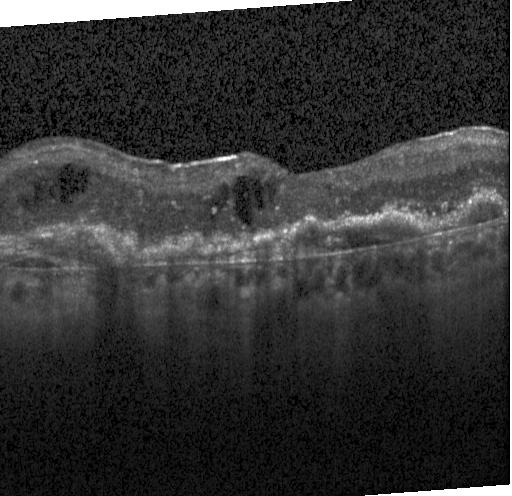

Assessment: a choroidal neovascular membrane.